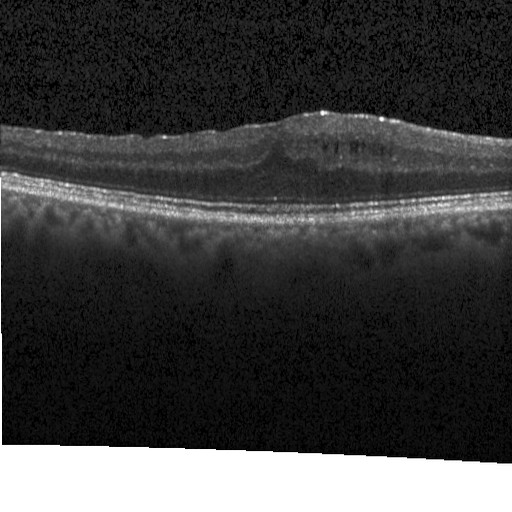

Spectral-domain optical coherence tomography. Heidelberg Spectralis. OCT B-scan.
Diabetic macular edema.